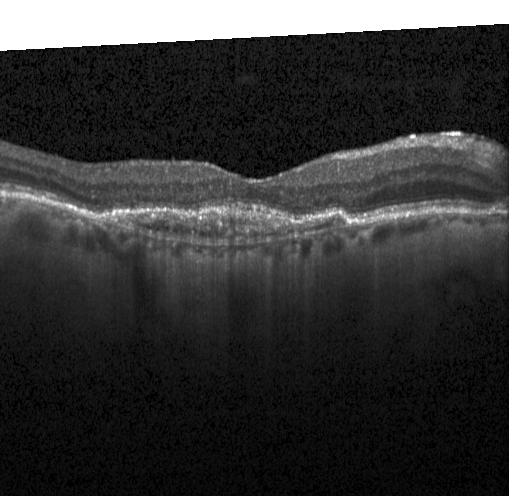

Optical coherence tomography B-scan
Choroidal neovascularization (CNV).